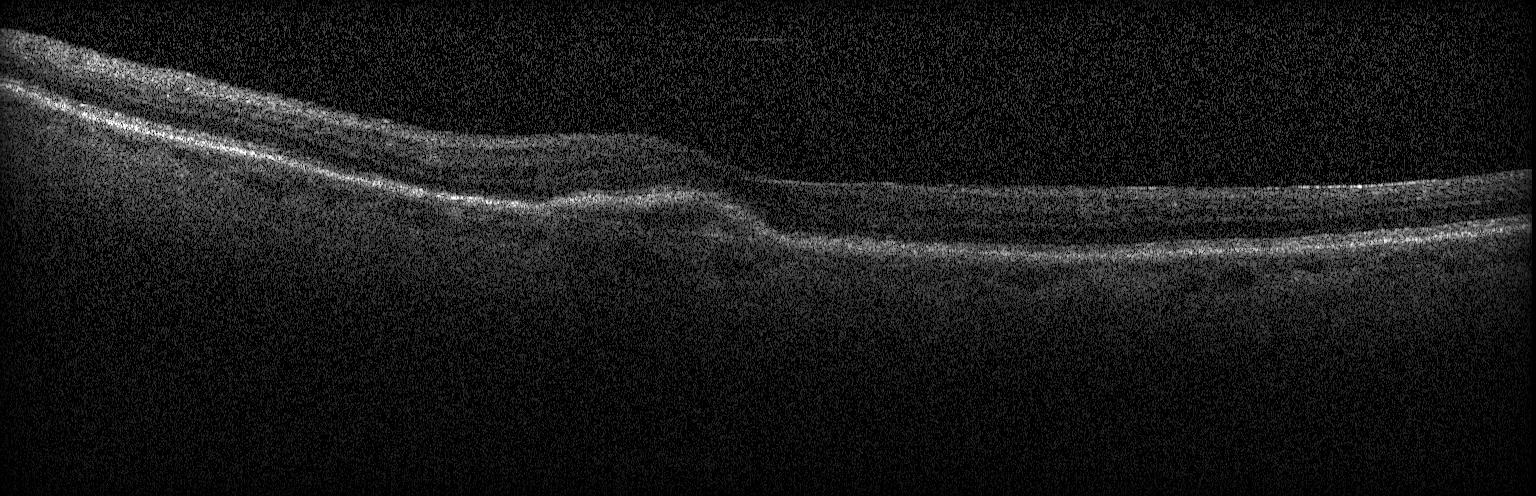 Optical coherence tomography B-scan; SD-OCT — This B-scan demonstrates choroidal neovascularization.